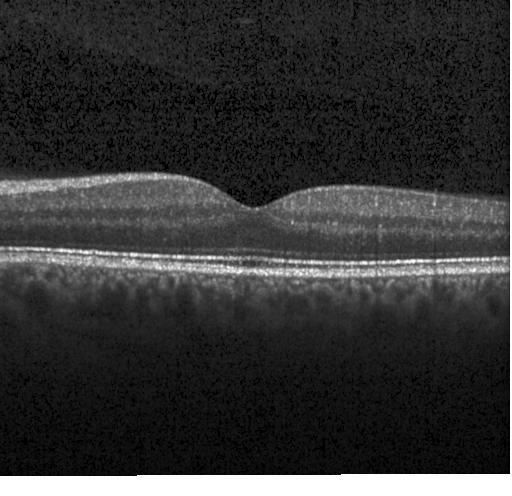

OCT finding: no evidence of choroidal neovascularization, diabetic macular edema, or drusen.